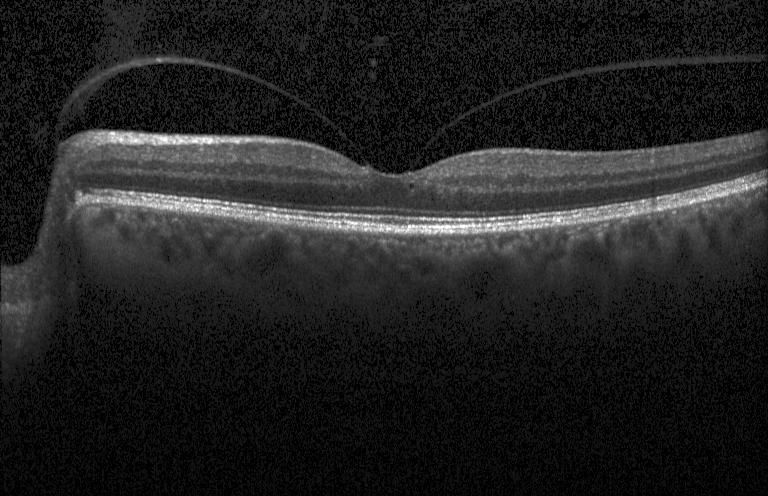

Finding: no CNV, DME, or drusen.